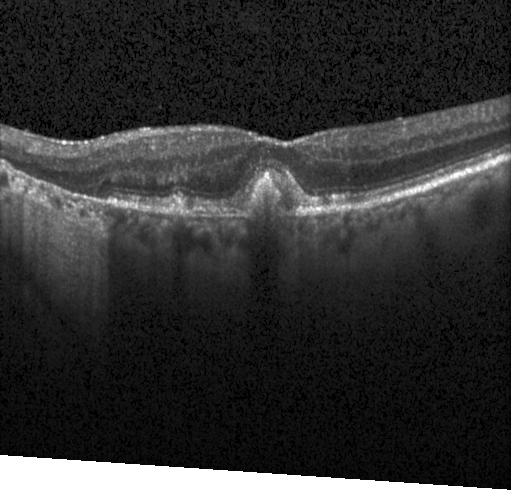 Spectral-domain OCT B-scan: a choroidal neovascular membrane.